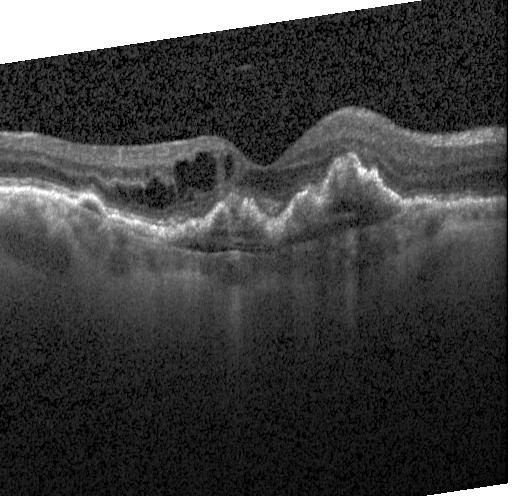
Optical coherence tomography scan; acquired on a Heidelberg Spectralis; SD-OCT; macular scan — OCT finding: choroidal neovascularization (CNV).